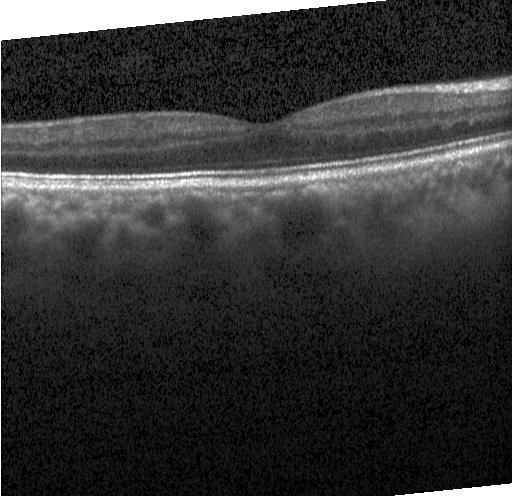 Spectral-domain OCT · optical coherence tomography scan
Macular OCT: no evidence of CNV, DME, or drusen.